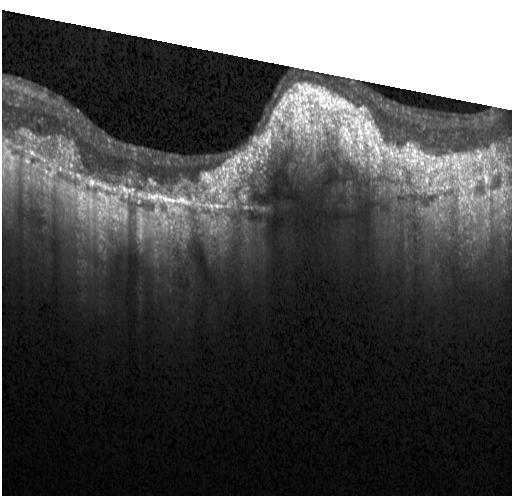
OCT B-scan. Impression: a choroidal neovascular membrane.